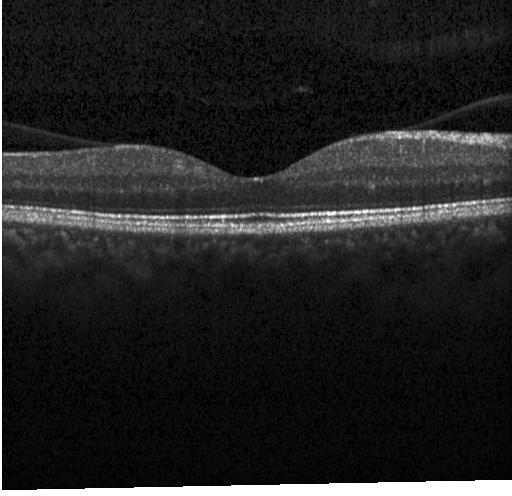

Dx: no CNV, no DME, and no drusen.